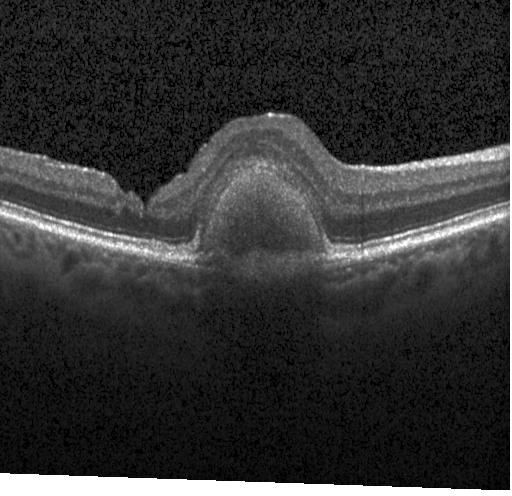

Macular OCT: a choroidal neovascular membrane.